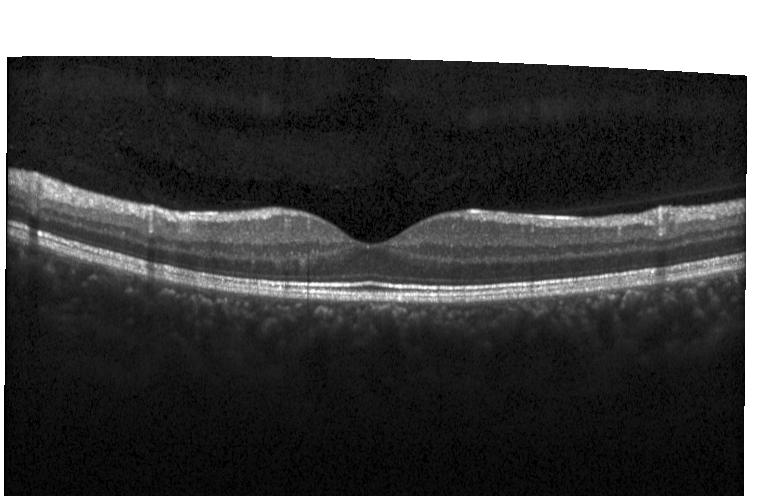

OCT B-scan · centered on the fovea · SD-OCT
Finding: neither CNV, DME, nor drusen.